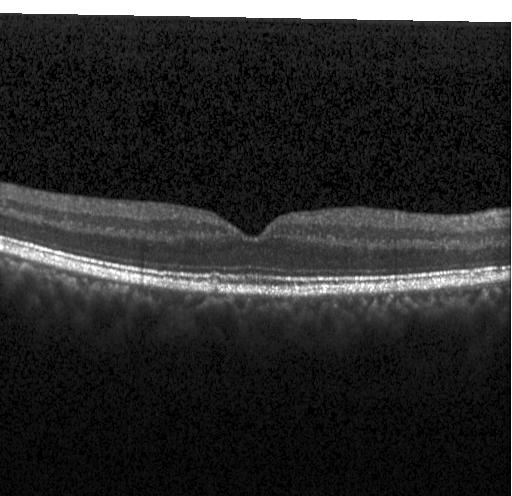
Acquired on a Heidelberg Spectralis · retinal OCT cross-section. No choroidal neovascularization, diabetic macular edema, or drusen.